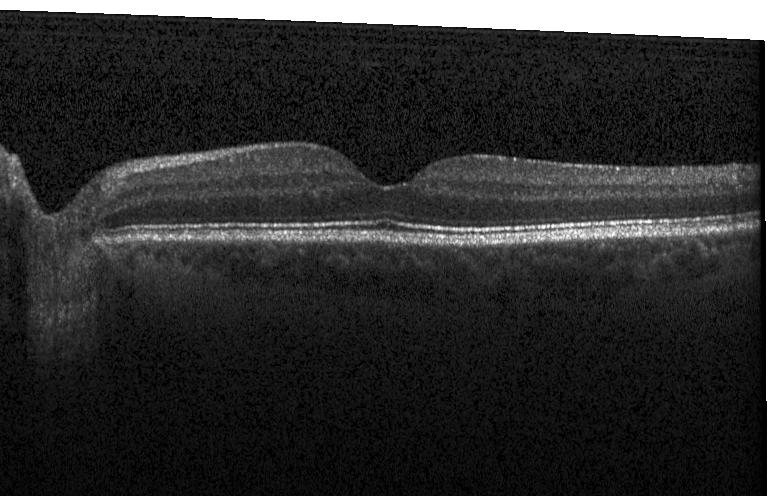

Spectral-domain optical coherence tomography. OCT line scan — Impression: no evidence of choroidal neovascularization, diabetic macular edema, or drusen.